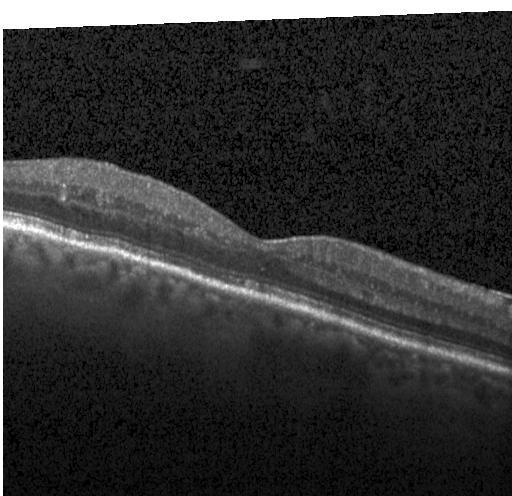 Spectral-domain OCT B-scan: no CNV, no DME, and no drusen.